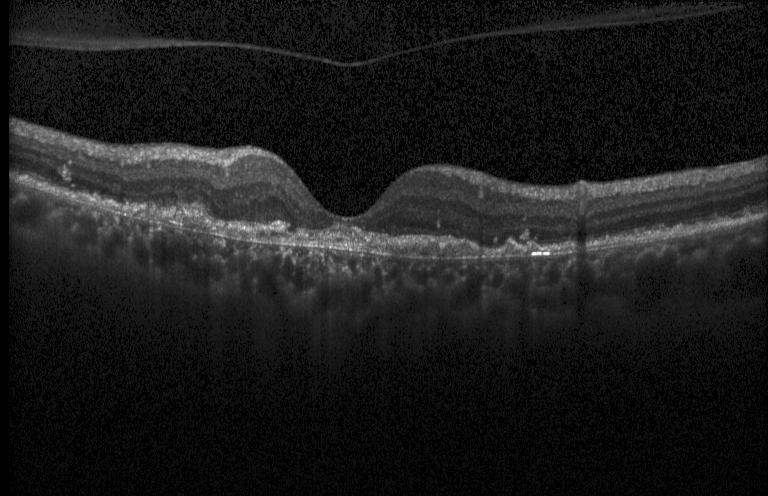 Optical coherence tomography B-scan · SD-OCT.
Diagnosis: a choroidal neovascular membrane.